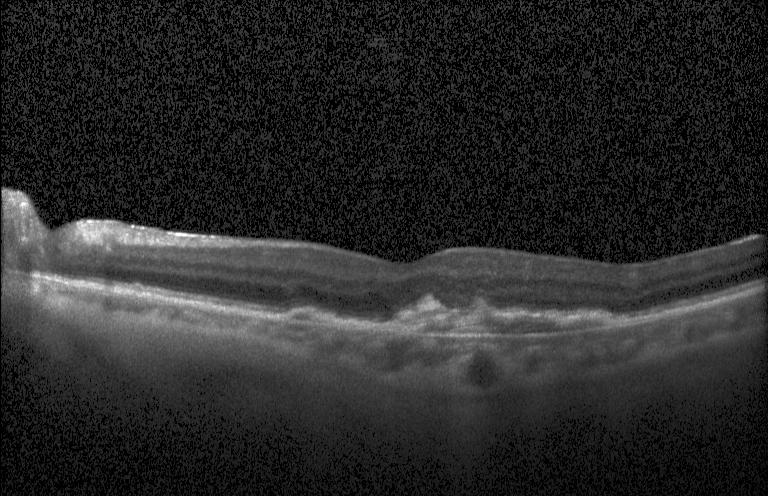
Optical coherence tomography B-scan, SD-OCT — The scan shows a choroidal neovascular membrane.